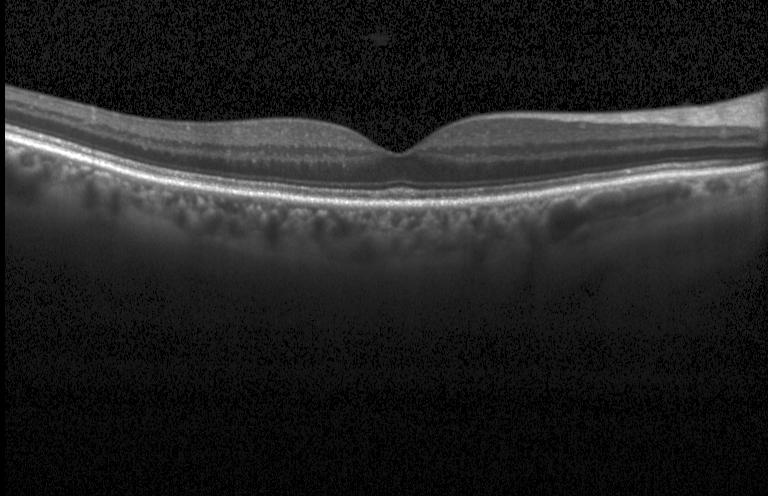

Fovea-centered; SD-OCT; optical coherence tomography scan; Heidelberg Spectralis OCT system. Macular OCT: no evidence of CNV, DME, or drusen.